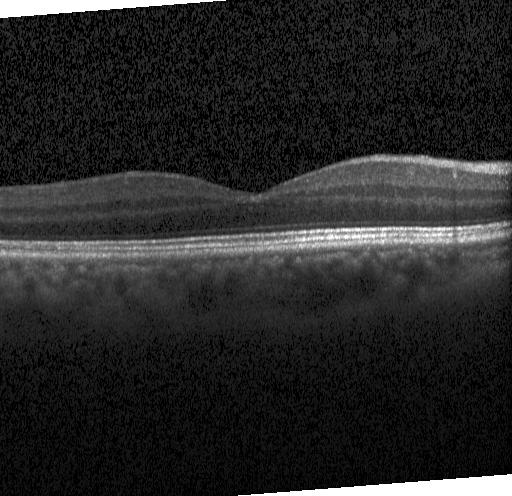 Optical coherence tomography scan. Instrument: Heidelberg Spectralis. Horizontal scan through the fovea.
The scan shows no CNV, DME, or drusen.